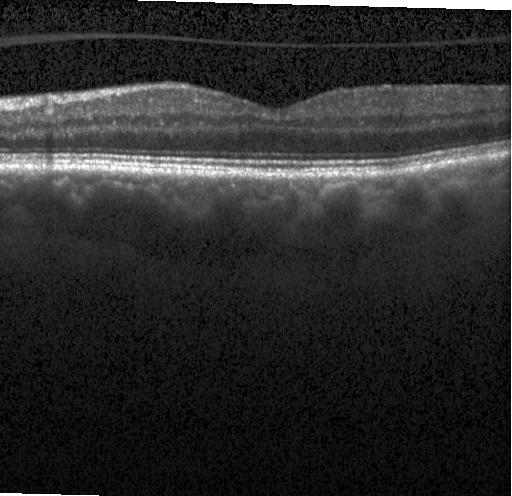 Spectral-domain OCT, fovea-centered, instrument: Heidelberg Spectralis, retinal OCT B-scan — Impression: no choroidal neovascularization, no diabetic macular edema, and no drusen.